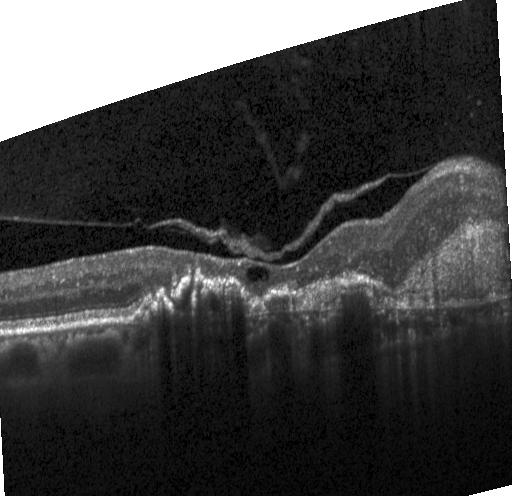

Through the macula; Heidelberg Spectralis; retinal OCT B-scan
Dx: CNV.